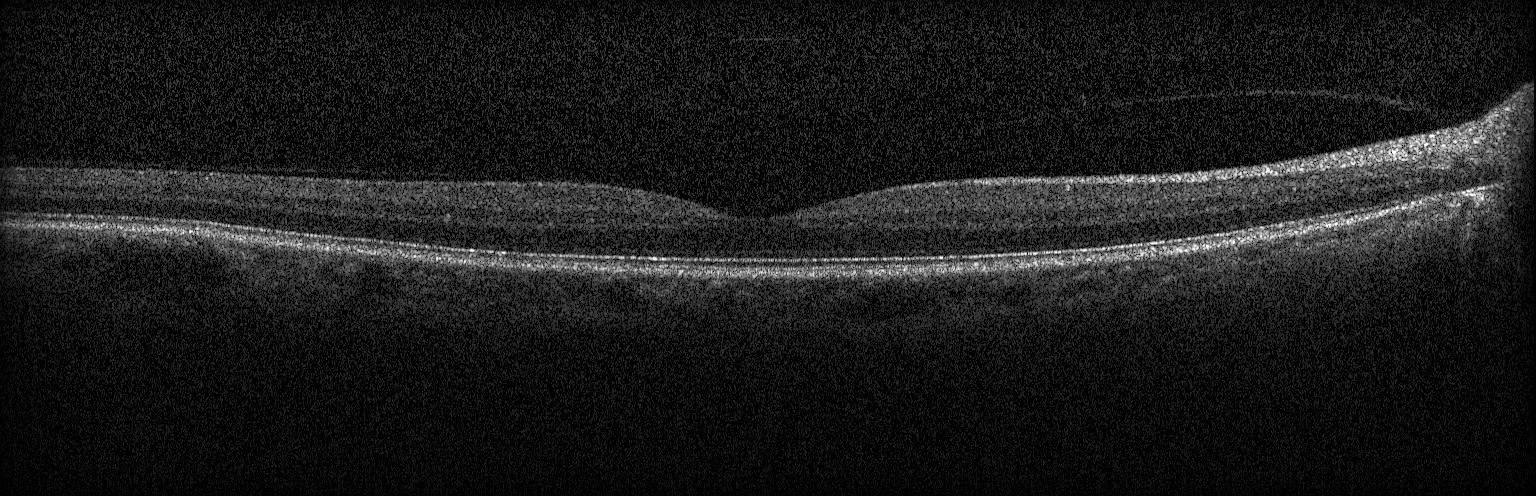
Instrument: Heidelberg Spectralis · spectral-domain optical coherence tomography · OCT line scan · through the macula
Impression: no evidence of choroidal neovascularization, diabetic macular edema, or drusen.